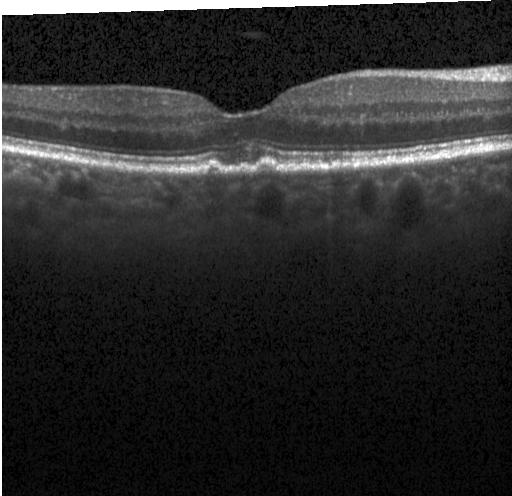
Optical coherence tomography B-scan. Centered on the fovea. Finding: multiple drusen.